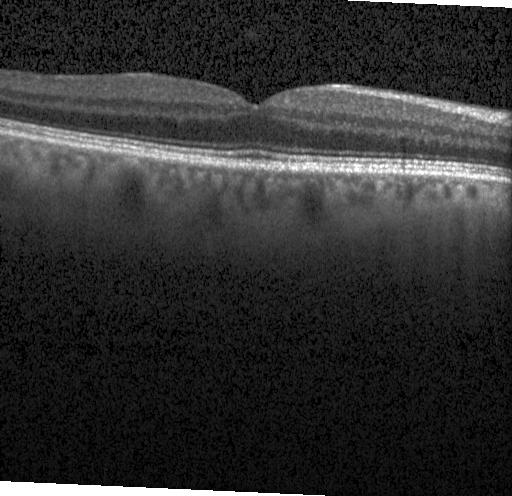 Retinal OCT B-scan; fovea-centered; acquired on a Heidelberg Spectralis; spectral-domain OCT.
Impression: no evidence of CNV, DME, or drusen.